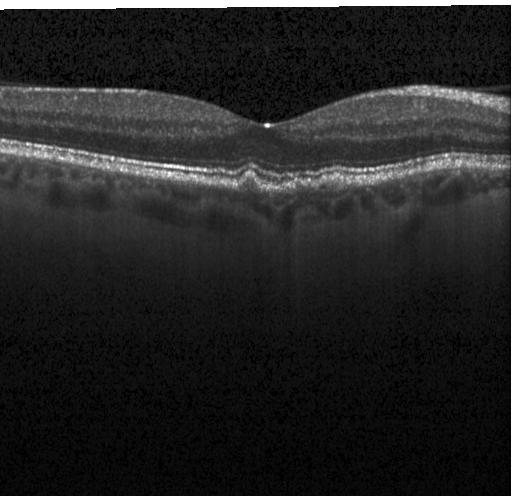

Finding: sub-RPE drusenoid deposits.